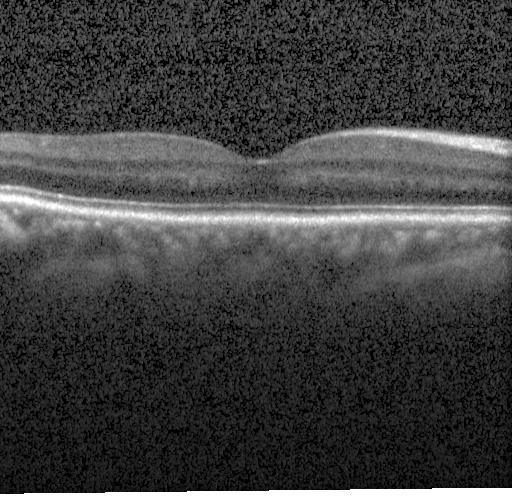

OCT B-scan showing no choroidal neovascularization, no diabetic macular edema, and no drusen.